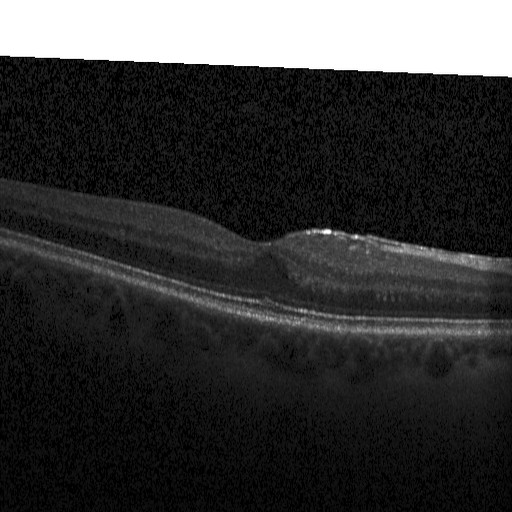

OCT line scan; horizontal scan through the fovea; spectral-domain optical coherence tomography; instrument: Heidelberg Spectralis — Dx: diabetic macular edema (DME).